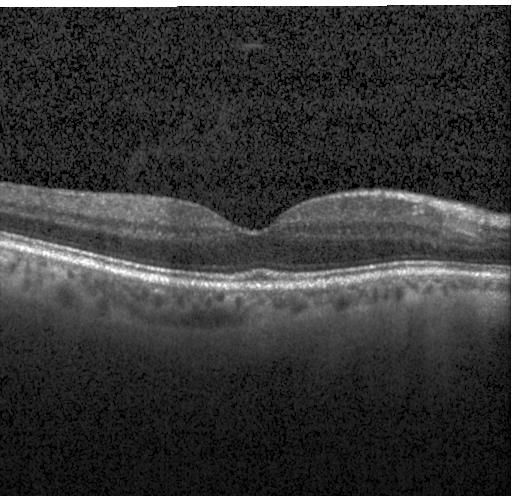 OCT finding: no evidence of choroidal neovascularization, diabetic macular edema, or drusen.